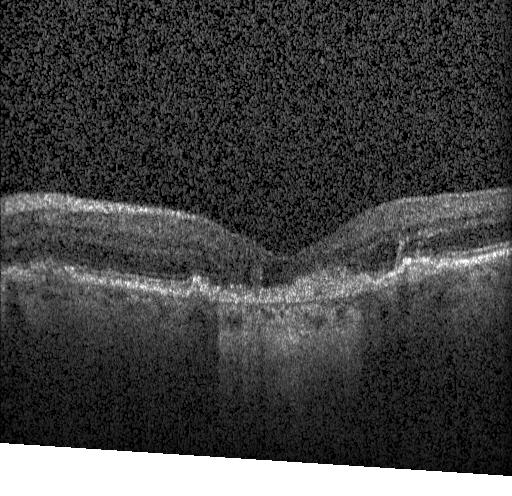
Spectral-domain OCT, acquired on a Heidelberg Spectralis, OCT line scan, horizontal scan through the fovea — This B-scan demonstrates choroidal neovascularization.